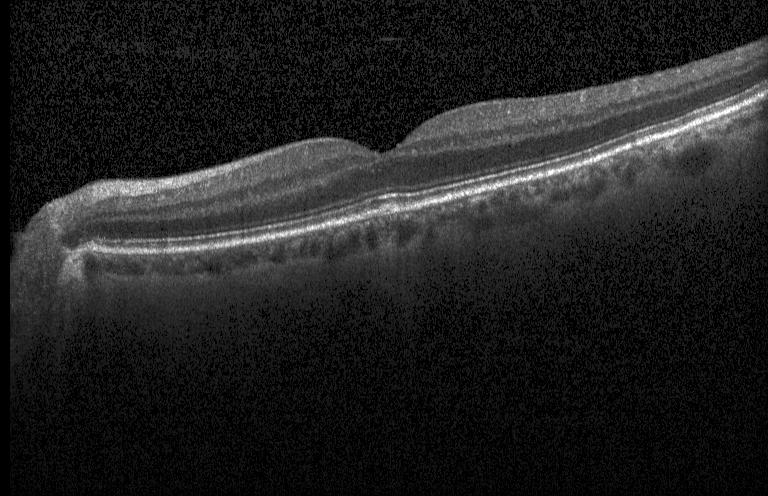

Dx: no choroidal neovascularization, diabetic macular edema, or drusen.